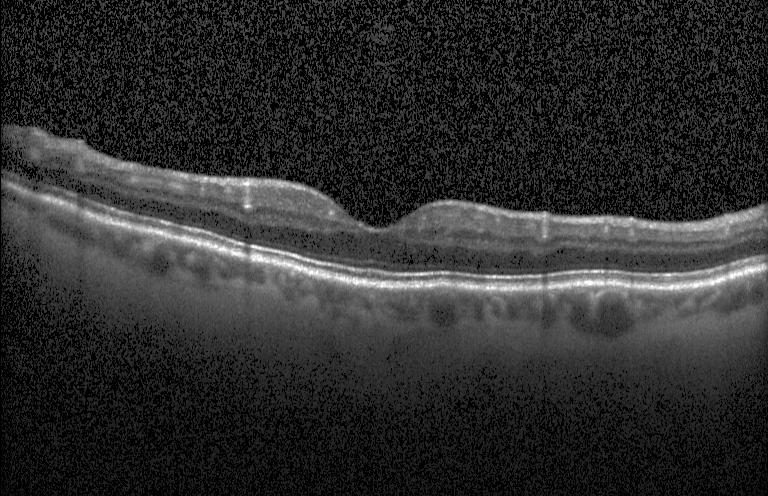
OCT scan showing neither CNV, DME, nor drusen.